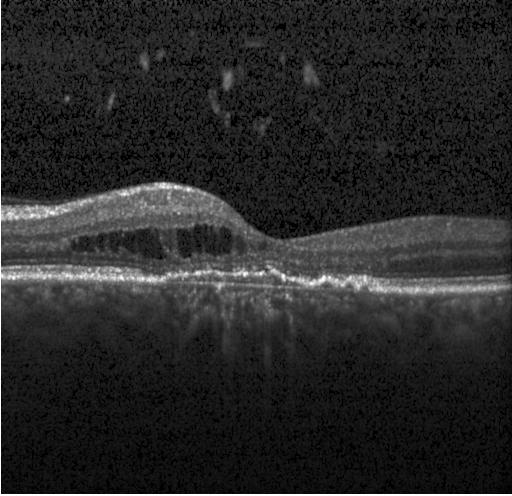

Retinal OCT B-scan · macular scan · SD-OCT · Heidelberg Spectralis OCT system — Dx: a choroidal neovascular membrane.